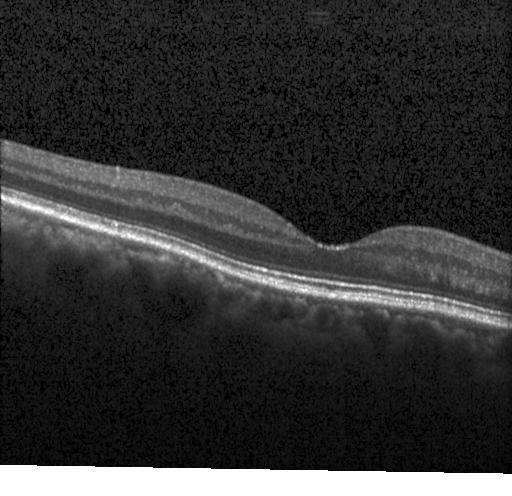 Diagnosis: no CNV, no DME, and no drusen.